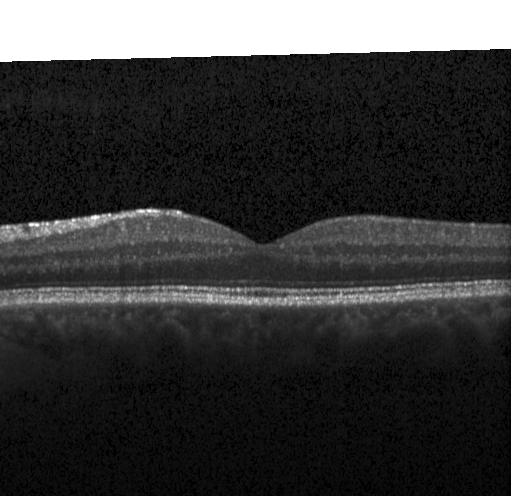

Retinal OCT cross-section
No choroidal neovascularization, no diabetic macular edema, and no drusen.